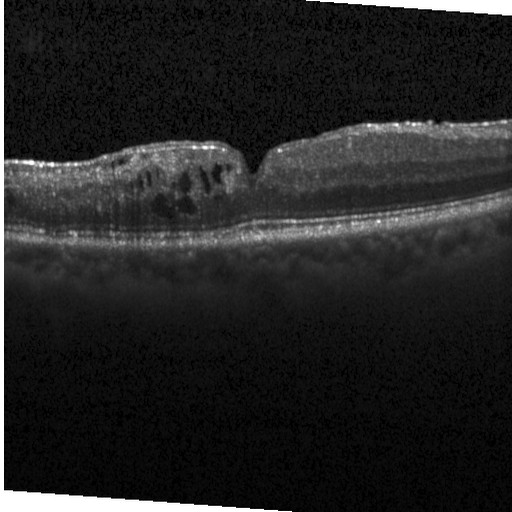 Spectral-domain optical coherence tomography, instrument: Heidelberg Spectralis, fovea-centered, retinal OCT B-scan. Finding: DME.